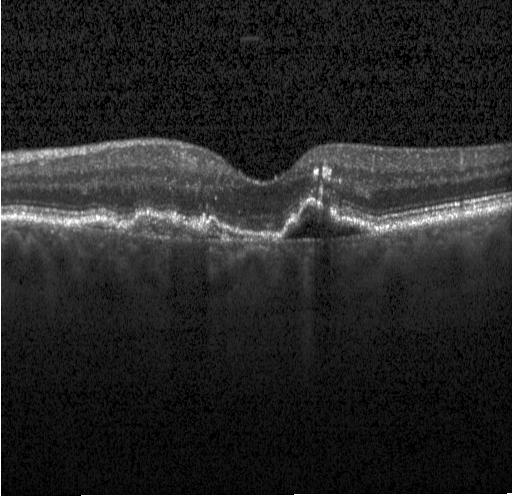

Optical coherence tomography B-scan, macular scan, spectral-domain OCT, acquired on a Heidelberg Spectralis
Assessment: a choroidal neovascular membrane.